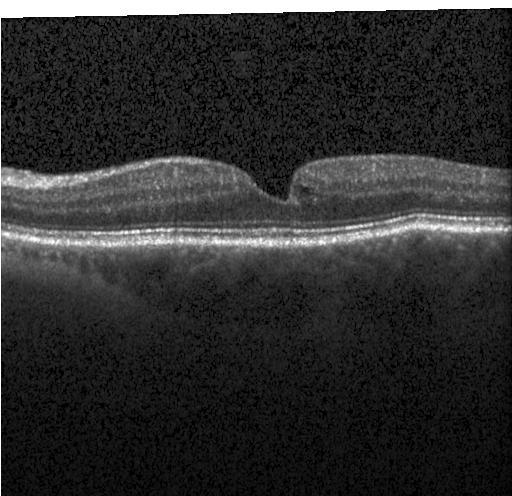
Heidelberg Spectralis; OCT line scan; horizontal scan through the fovea; spectral-domain optical coherence tomography. Diabetic macular edema.